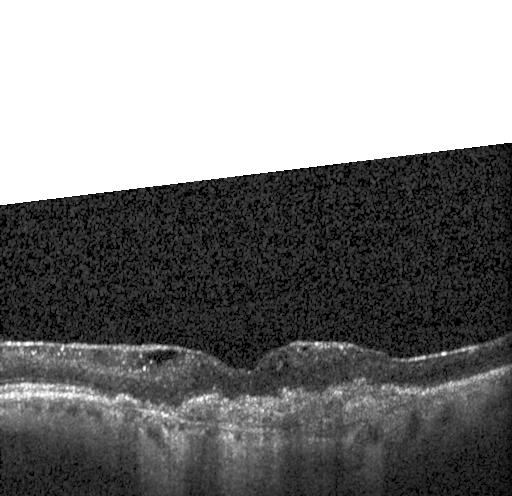

Finding: a choroidal neovascular membrane.